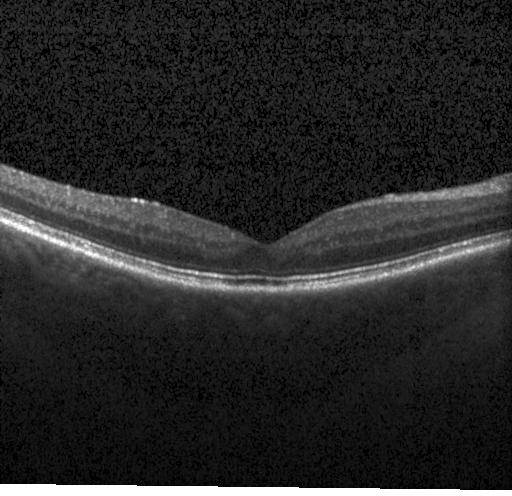

SD-OCT. Retinal OCT B-scan.
Diagnosis: no choroidal neovascularization, no diabetic macular edema, and no drusen.